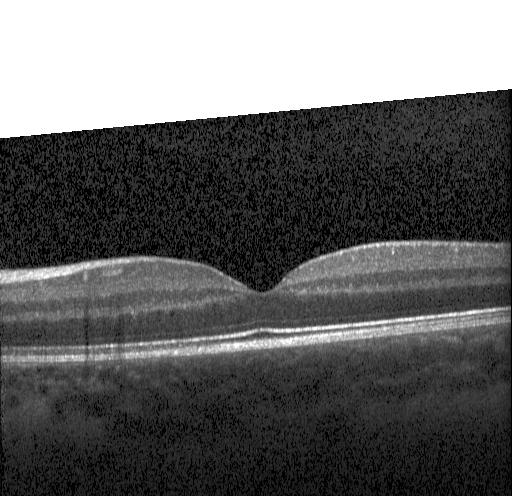

OCT B-scan
Diagnosis: no choroidal neovascularization, diabetic macular edema, or drusen.